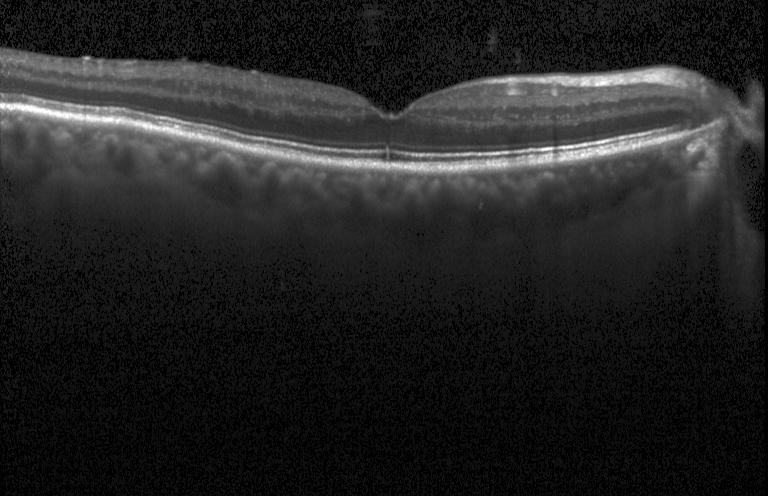

Retinal OCT cross-section — Impression: no choroidal neovascularization, diabetic macular edema, or drusen.